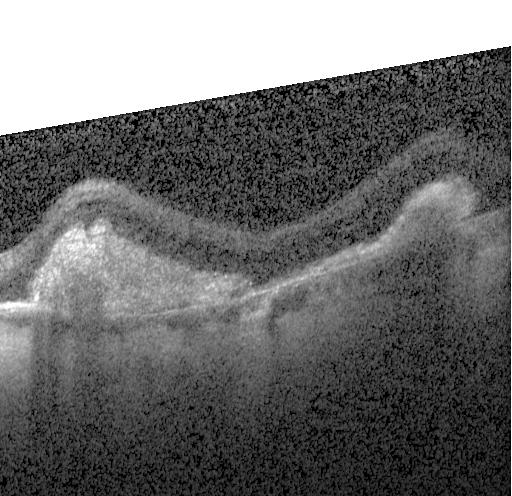
Macular OCT: a choroidal neovascular membrane.